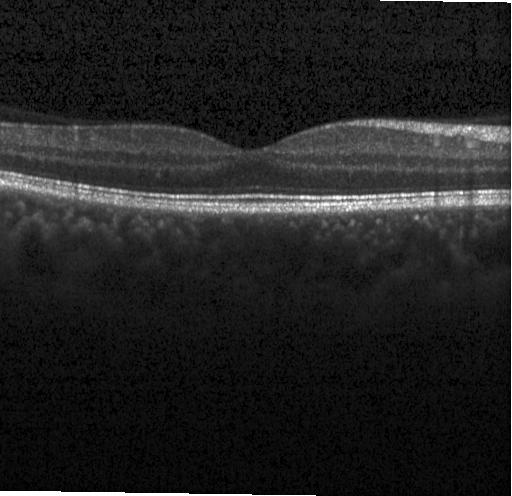
Optical coherence tomography scan · SD-OCT
Finding: no evidence of choroidal neovascularization, diabetic macular edema, or drusen.